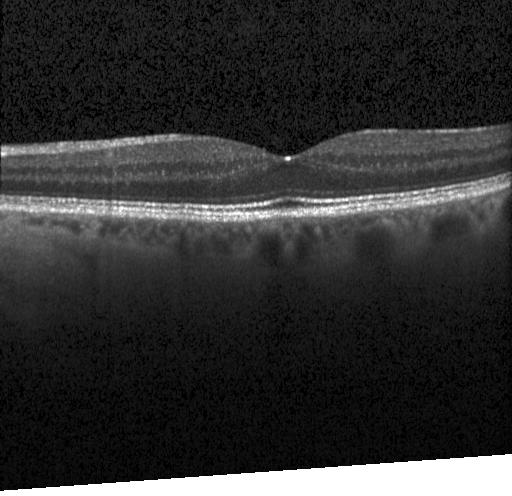
Retinal OCT B-scan. Fovea-centered
Finding: no CNV, no DME, and no drusen.